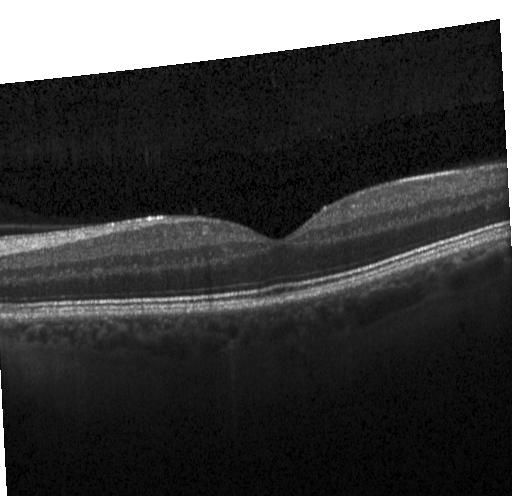

Through the macula, retinal OCT B-scan — Macular OCT: no choroidal neovascularization, diabetic macular edema, or drusen.